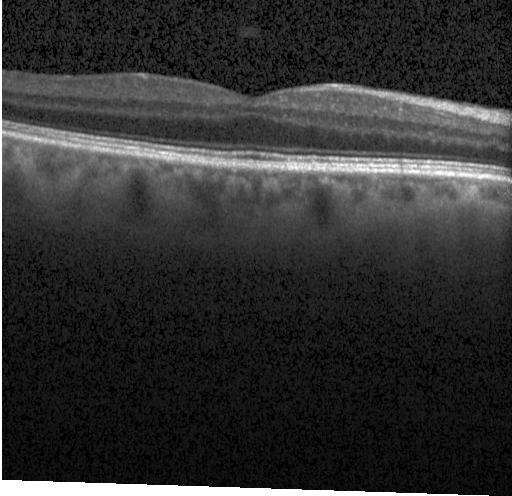
OCT B-scan showing no CNV, no DME, and no drusen.